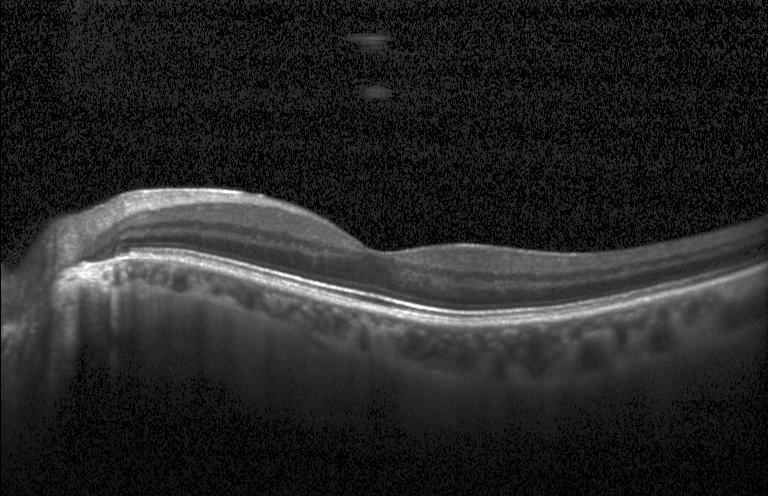
Macular scan; acquired on a Heidelberg Spectralis; OCT line scan; SD-OCT. No choroidal neovascularization, diabetic macular edema, or drusen.